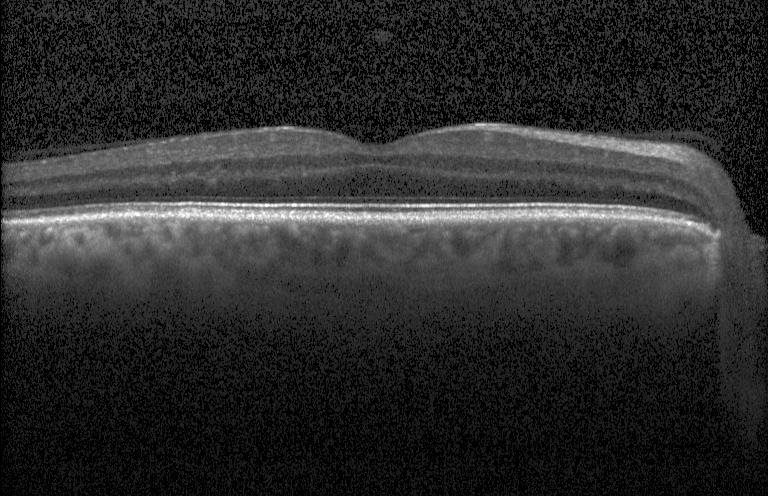
Retinal OCT B-scan, centered on the fovea, spectral-domain optical coherence tomography, Heidelberg Spectralis.
Dx: neither CNV, DME, nor drusen.